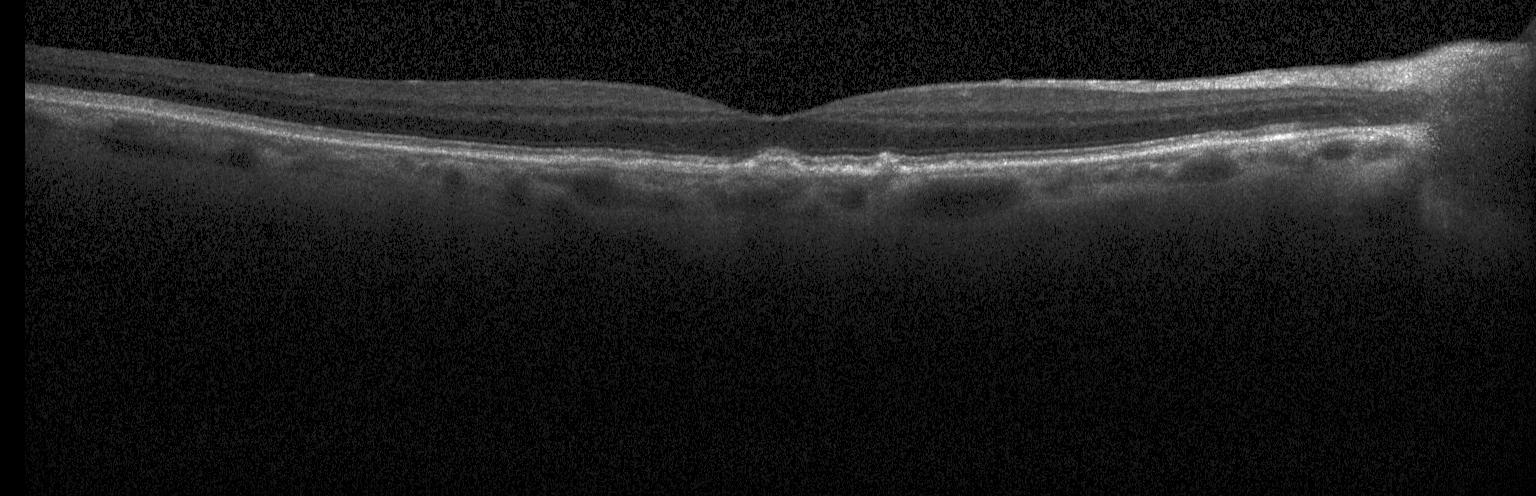 Optical coherence tomography scan — This B-scan demonstrates drusen.